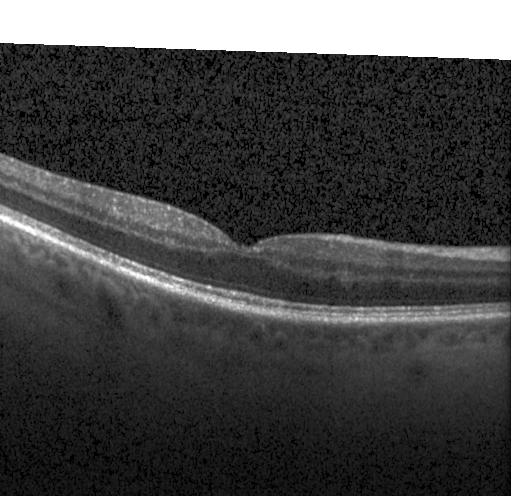
Macular OCT: no evidence of choroidal neovascularization, diabetic macular edema, or drusen.